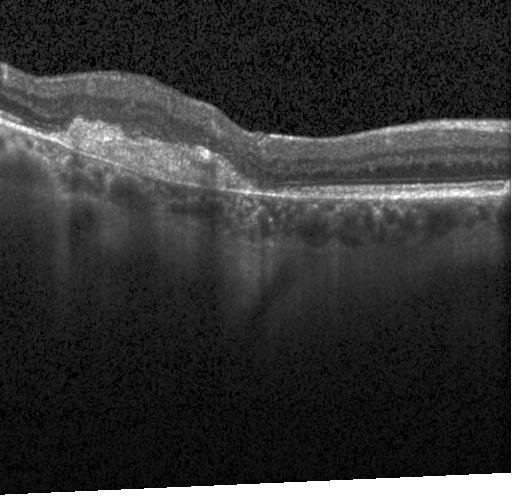 Impression: a choroidal neovascular membrane.